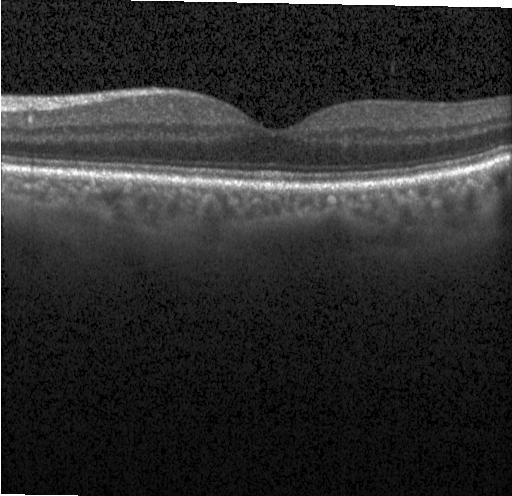

Retinal OCT B-scan. Macular scan.
Assessment: no evidence of choroidal neovascularization, diabetic macular edema, or drusen.